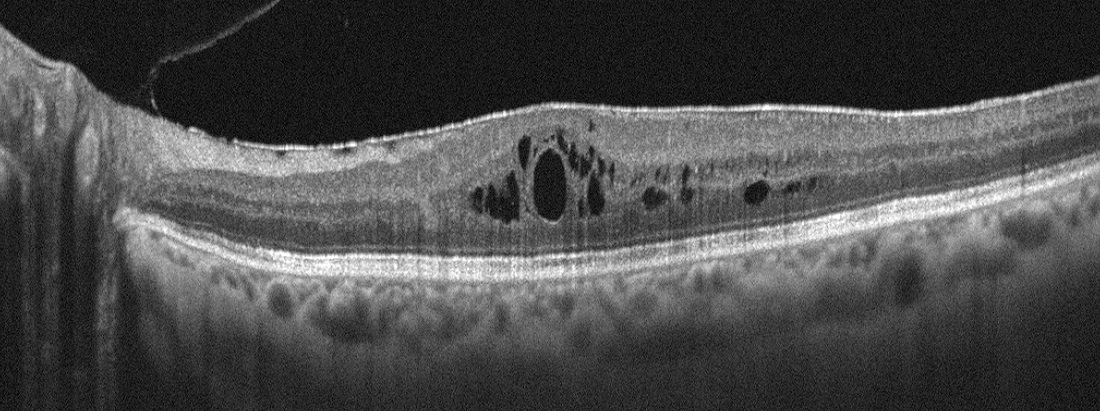
Through the macula; OCT line scan; Optovue Avanti RTVue XR. Epiretinal membrane (ERM).